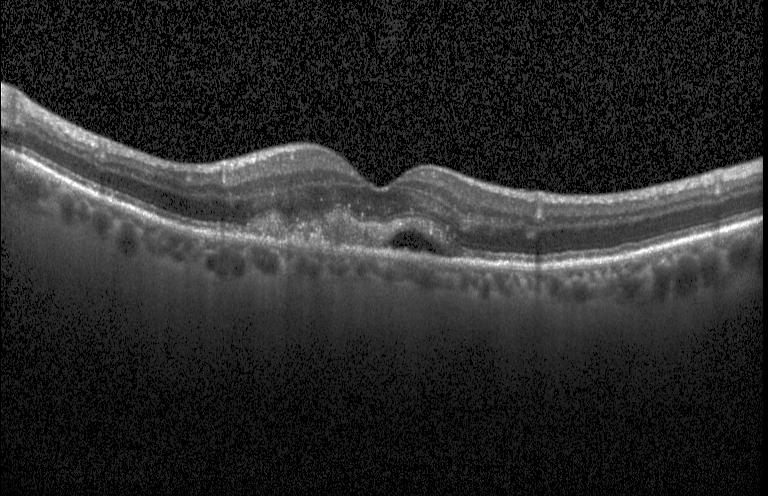

This B-scan demonstrates a choroidal neovascular membrane.